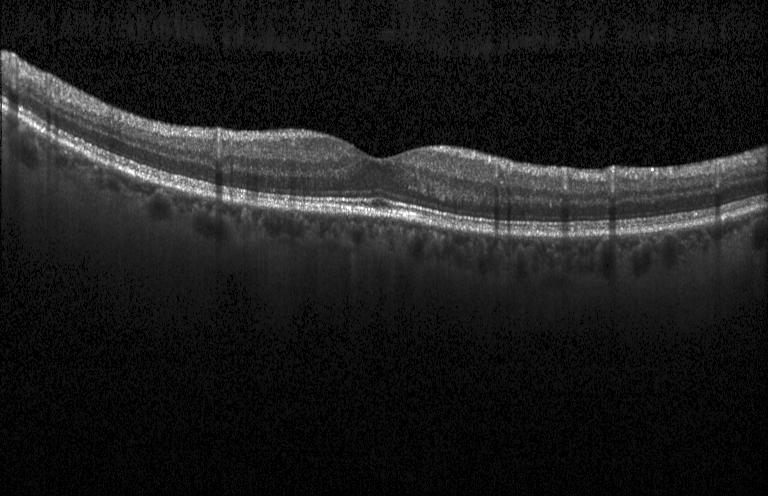

Spectral-domain OCT. Retinal OCT B-scan
OCT finding: no choroidal neovascularization, no diabetic macular edema, and no drusen.